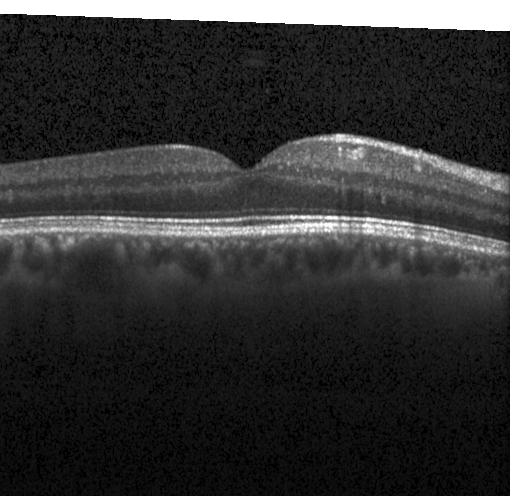

Heidelberg Spectralis · OCT B-scan · spectral-domain OCT · through the macula
Finding: no choroidal neovascularization, diabetic macular edema, or drusen.